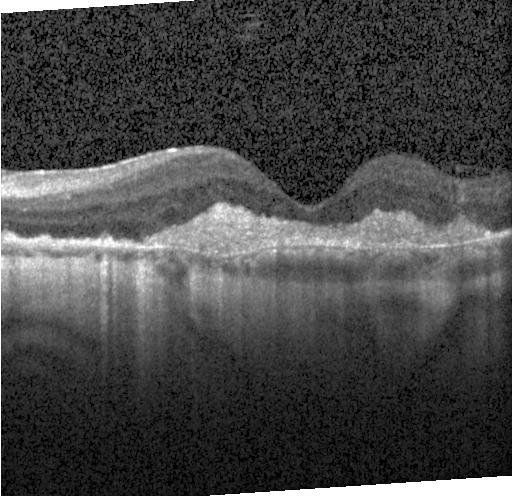
OCT line scan. Heidelberg Spectralis — Finding: choroidal neovascularization (CNV).